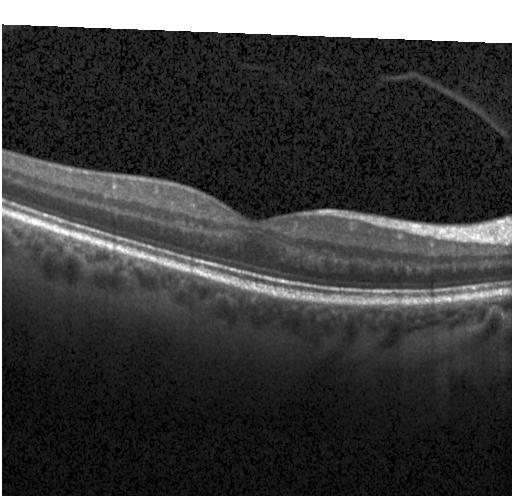

Centered on the fovea · acquired on a Heidelberg Spectralis · retinal OCT B-scan.
Diagnosis: no CNV, no DME, and no drusen.